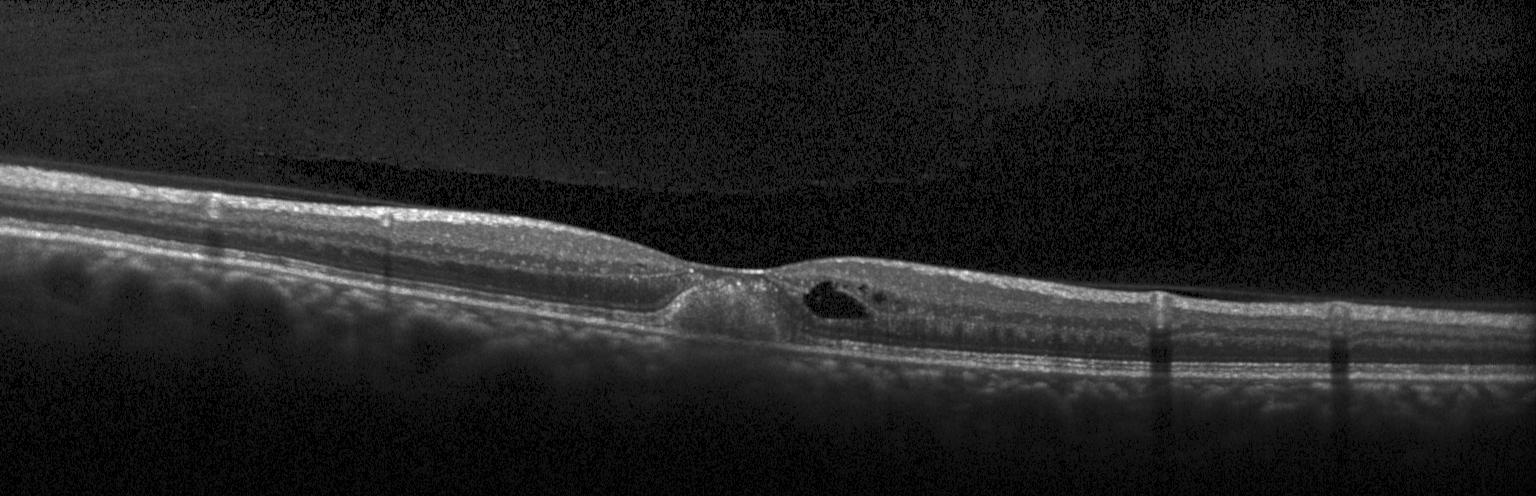

OCT finding: a choroidal neovascular membrane.